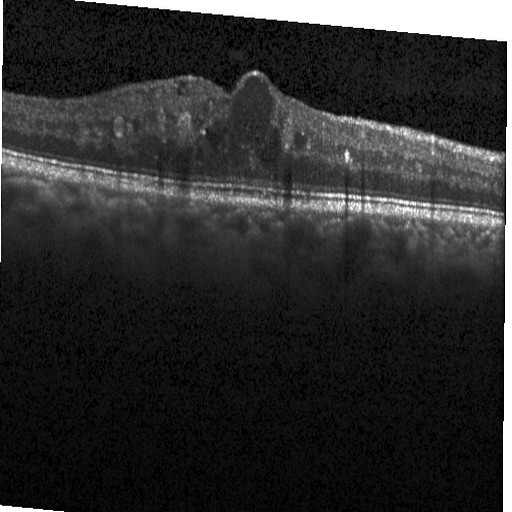 Macular scan; OCT B-scan — Finding: diabetic macular edema.